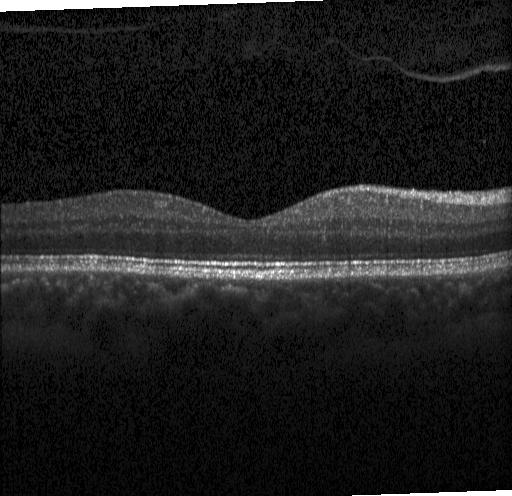

Optical coherence tomography B-scan — Assessment: no evidence of choroidal neovascularization, diabetic macular edema, or drusen.